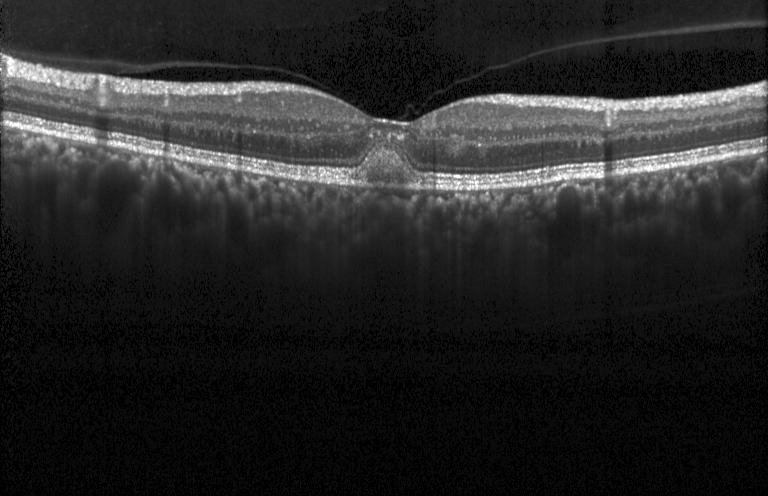
Choroidal neovascularization.